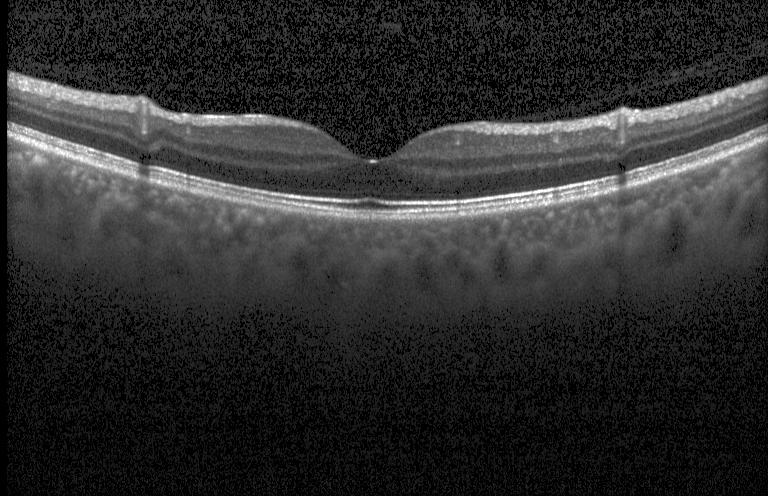 Macular OCT: no evidence of choroidal neovascularization, diabetic macular edema, or drusen.